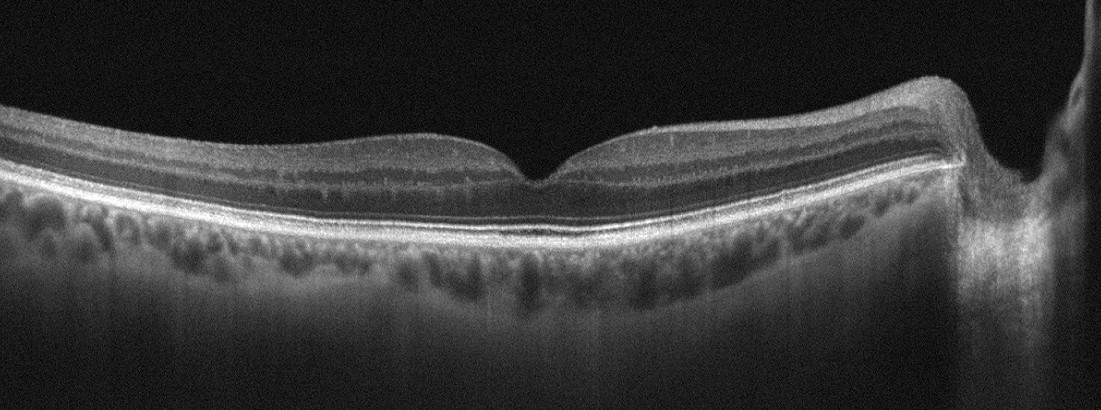 Macular scan. Optical coherence tomography B-scan. Instrument: Optovue Avanti RTVue XR — Impression: no evidence of AMD, DME, ERM, RAO, RVO, or VID.